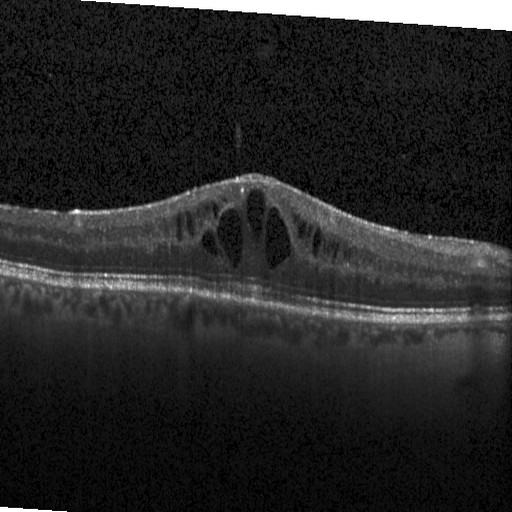
Spectral-domain OCT · OCT line scan · acquired on a Heidelberg Spectralis — Diagnosis: diabetic macular edema (DME).